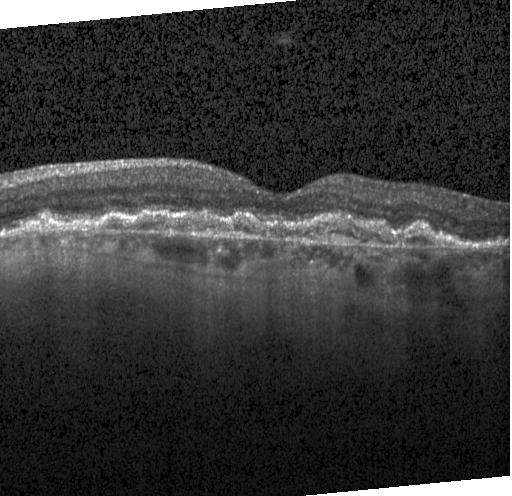

Fovea-centered. Retinal OCT cross-section.
This B-scan demonstrates a choroidal neovascular membrane.